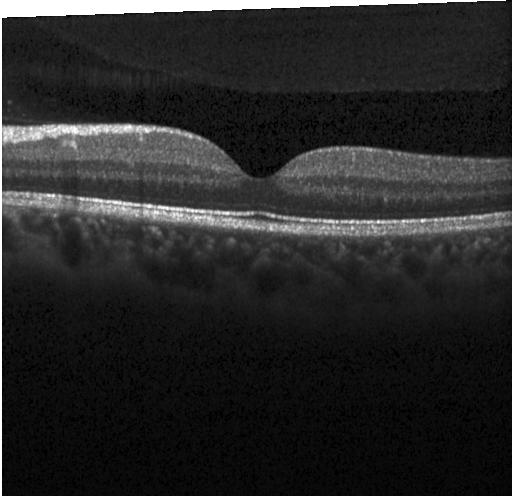
Through the macula. Optical coherence tomography scan. Heidelberg Spectralis OCT system. Spectral-domain OCT.
Finding: no choroidal neovascularization, diabetic macular edema, or drusen.